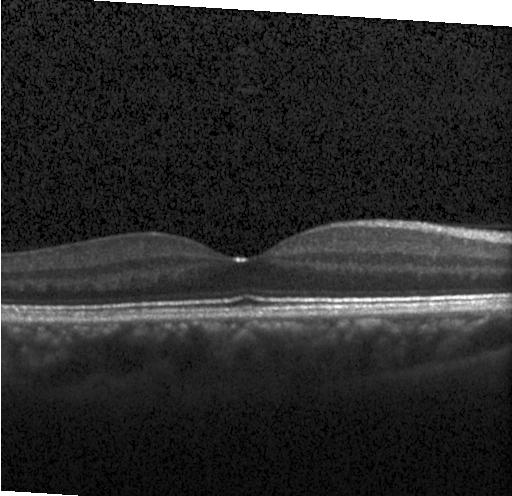
OCT line scan
OCT finding: neither choroidal neovascularization, diabetic macular edema, nor drusen.